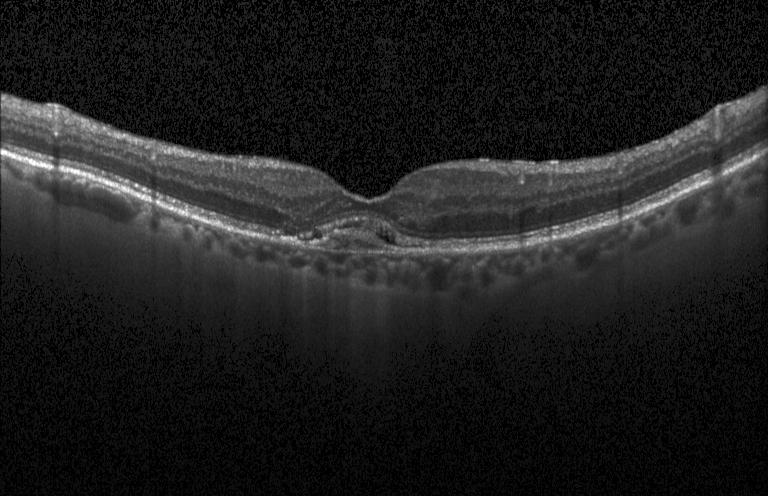
Macular OCT: a choroidal neovascular membrane.